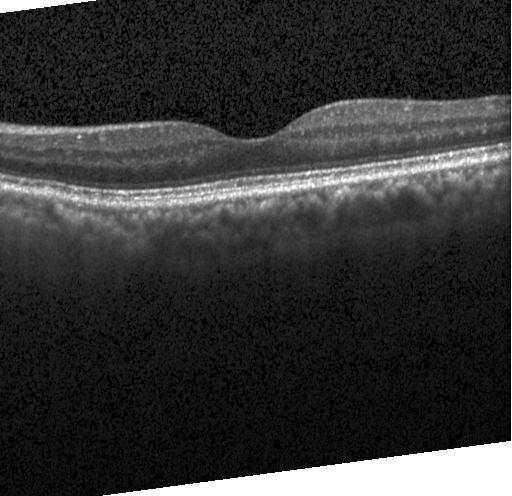
Optical coherence tomography scan; acquired on a Heidelberg Spectralis. Diagnosis: no evidence of choroidal neovascularization, diabetic macular edema, or drusen.